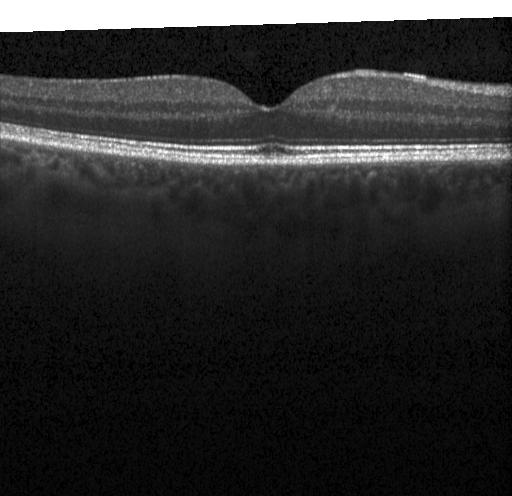

Retinal OCT cross-section.
Assessment: no CNV, DME, or drusen.